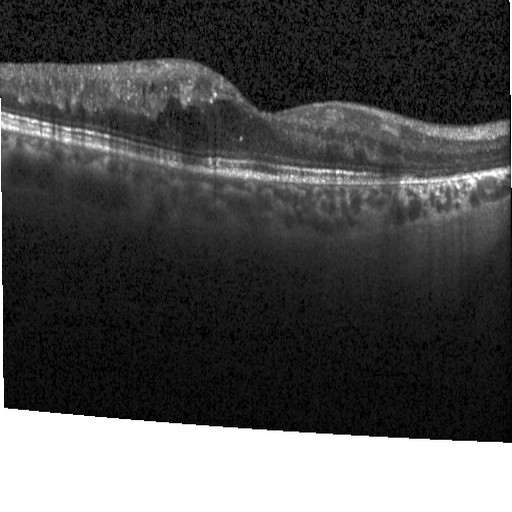
Retinal OCT B-scan — Impression: diabetic macular edema (DME).